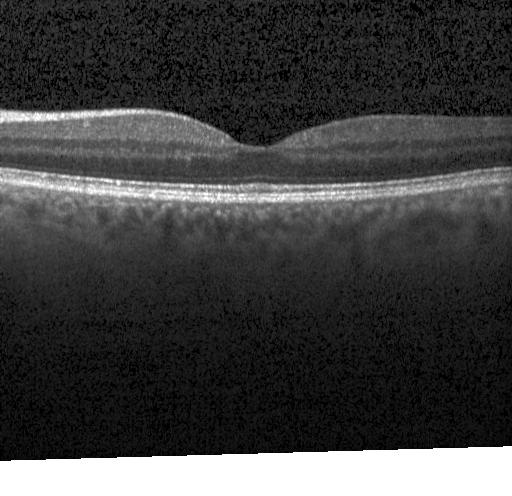

OCT line scan — Finding: neither choroidal neovascularization, diabetic macular edema, nor drusen.